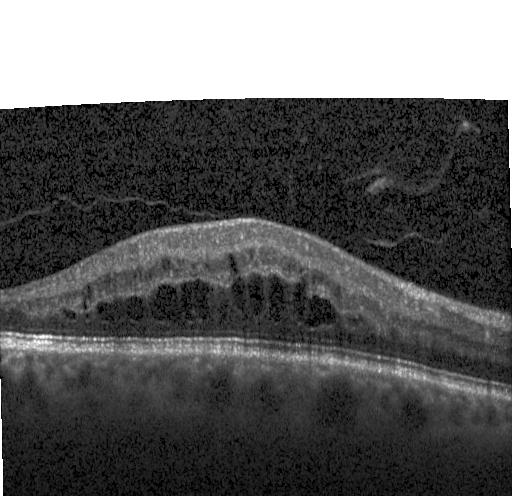
OCT scan showing diabetic macular edema (DME).